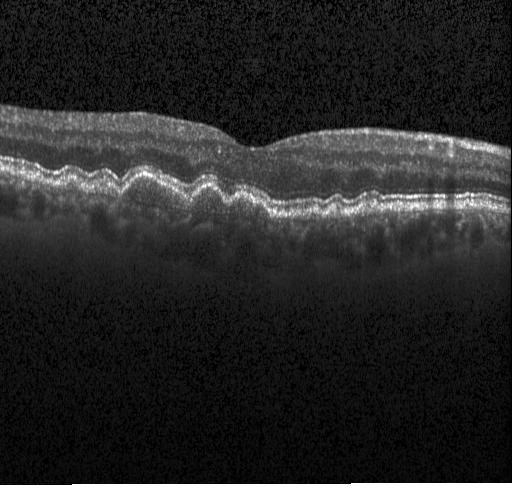

Finding: multiple drusen.